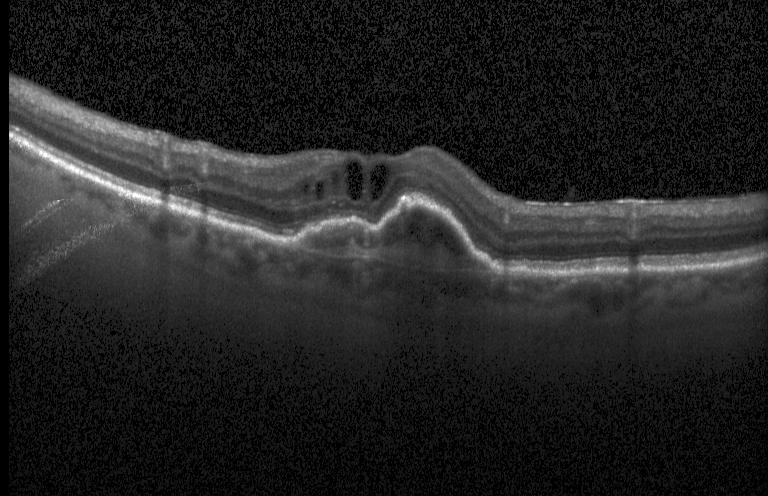

OCT B-scan.
Diagnosis: choroidal neovascularization.